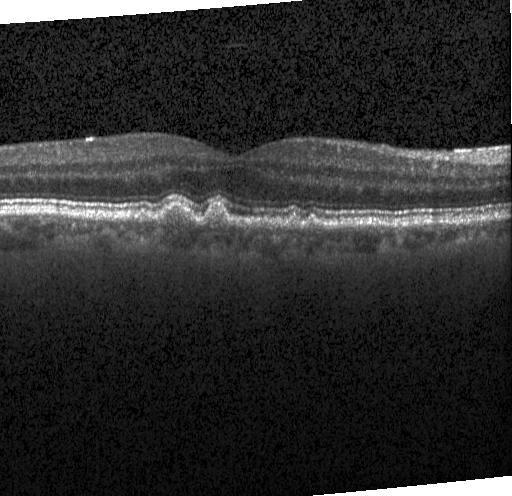
Finding: sub-RPE drusenoid deposits.